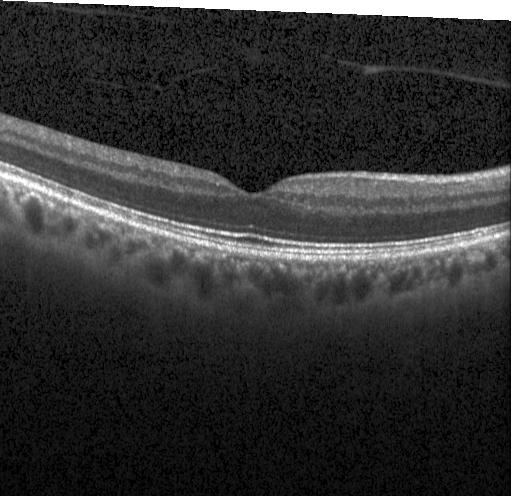
Retinal OCT cross-section, spectral-domain optical coherence tomography.
Assessment: neither choroidal neovascularization, diabetic macular edema, nor drusen.